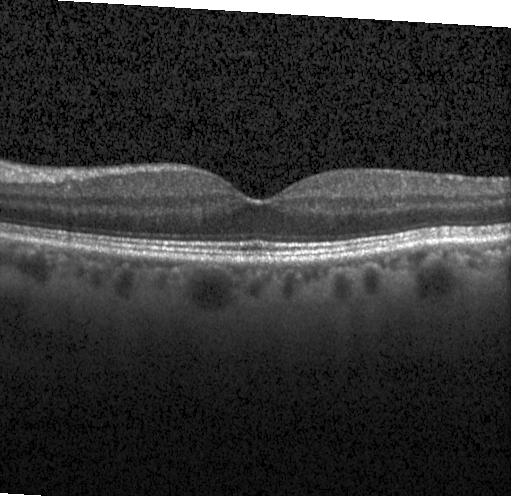

Retinal OCT B-scan.
This B-scan demonstrates no CNV, no DME, and no drusen.